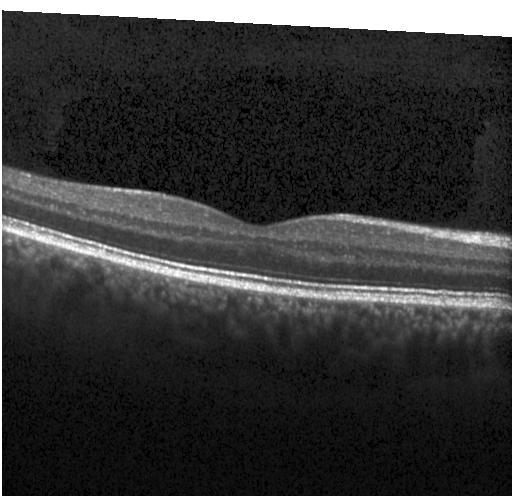

OCT finding: no choroidal neovascularization, no diabetic macular edema, and no drusen.